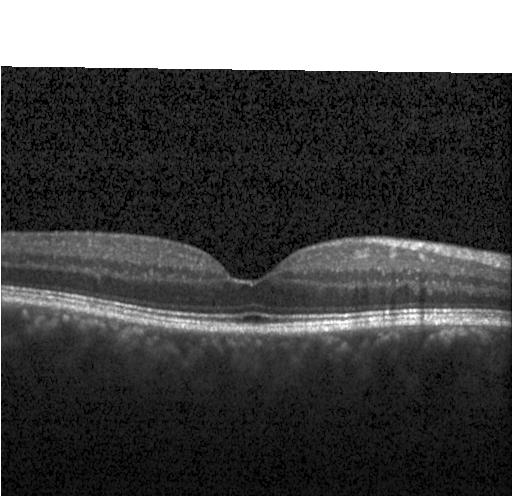 OCT line scan. Spectral-domain OCT.
Diagnosis: neither CNV, DME, nor drusen.